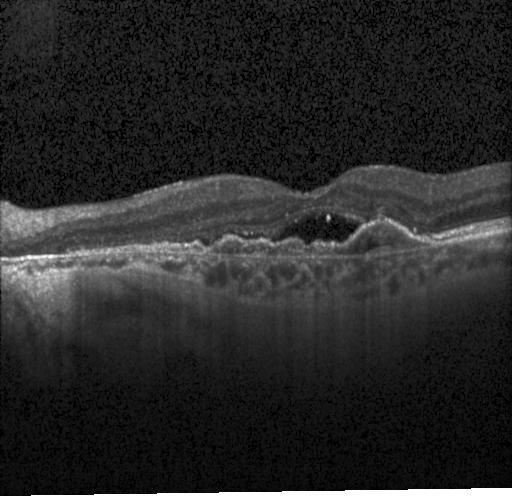 OCT B-scan.
Finding: a choroidal neovascular membrane.